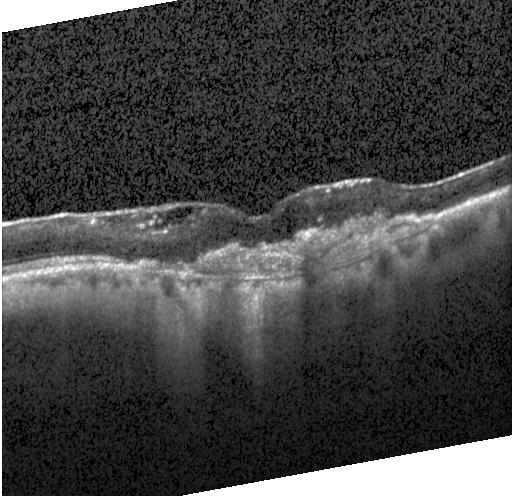

OCT line scan · Heidelberg Spectralis · spectral-domain optical coherence tomography · through the macula.
Finding: a choroidal neovascular membrane.